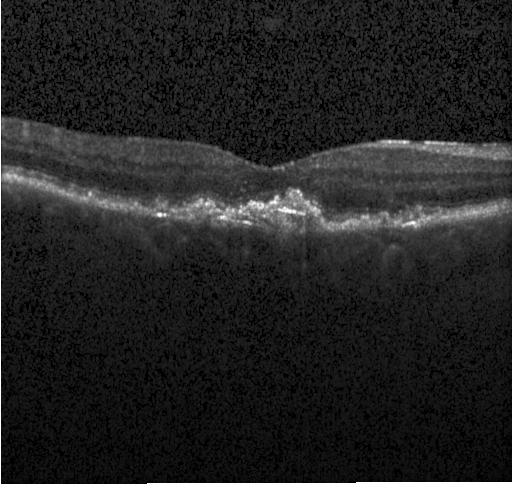

Spectral-domain OCT; optical coherence tomography B-scan.
The scan shows choroidal neovascularization (CNV).